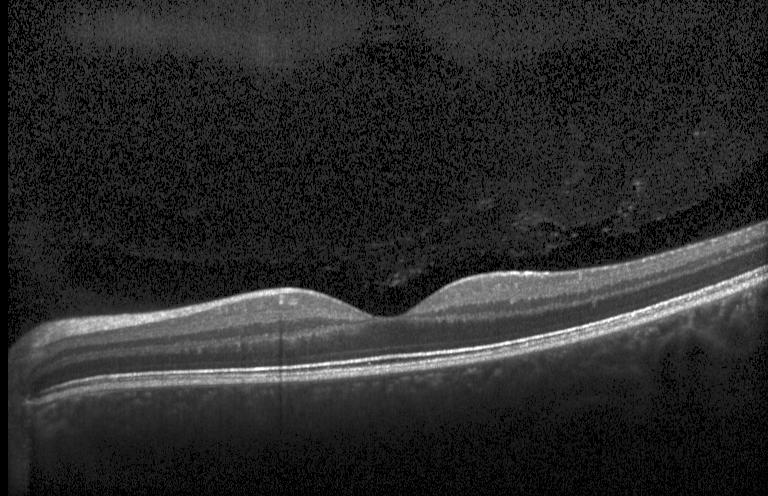 Macular OCT demonstrating no choroidal neovascularization, diabetic macular edema, or drusen.